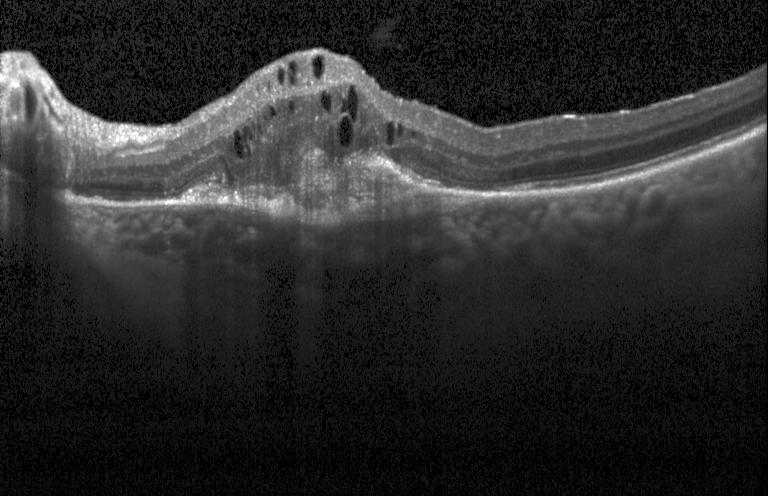

Optical coherence tomography scan; SD-OCT; Heidelberg Spectralis OCT system; fovea-centered
Impression: CNV.